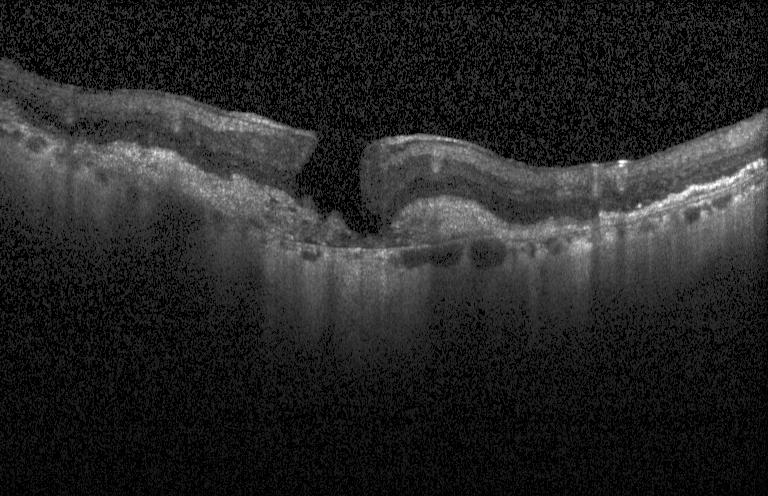

Retinal OCT cross-section · SD-OCT
OCT finding: choroidal neovascularization (CNV).